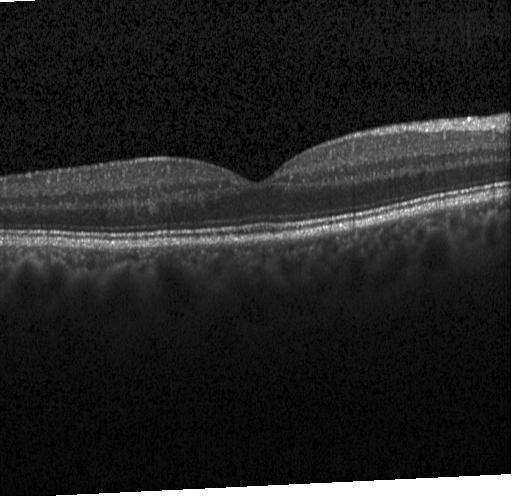
Instrument: Heidelberg Spectralis. Macular scan. Retinal OCT cross-section.
Assessment: no evidence of CNV, DME, or drusen.